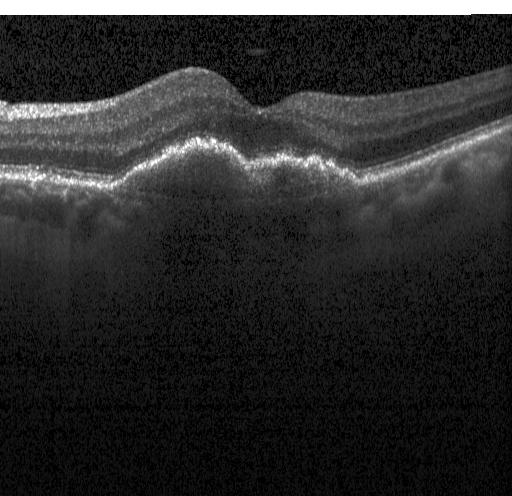 Retinal OCT cross-section showing a choroidal neovascular membrane.